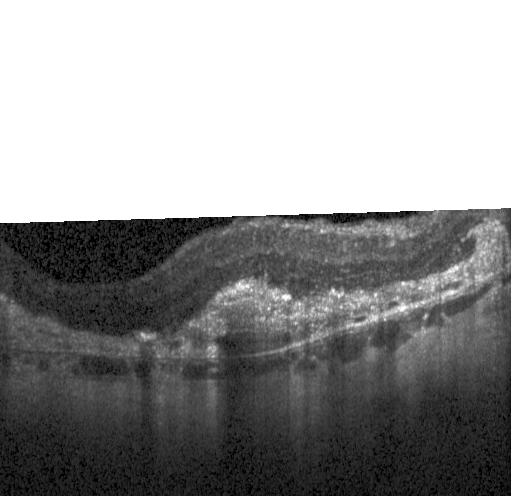

Heidelberg Spectralis; OCT B-scan.
Assessment: choroidal neovascularization (CNV).